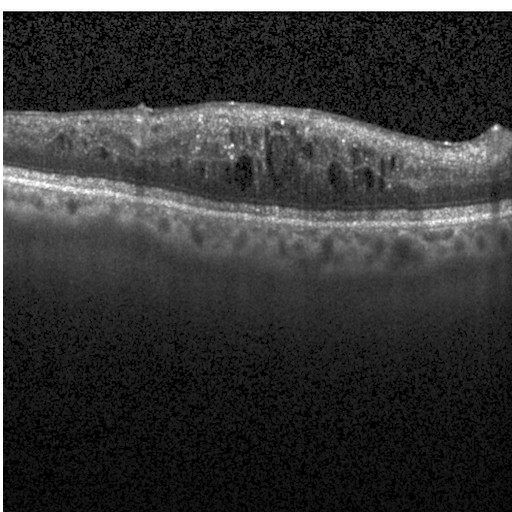 Spectral-domain OCT; macular scan; optical coherence tomography B-scan — This B-scan demonstrates diabetic macular edema.